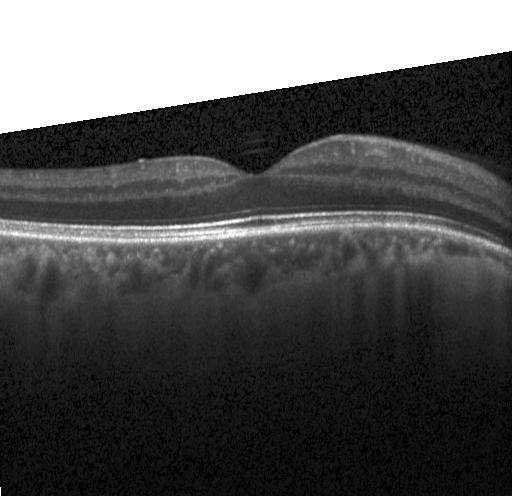

Macular OCT demonstrating no choroidal neovascularization, diabetic macular edema, or drusen.